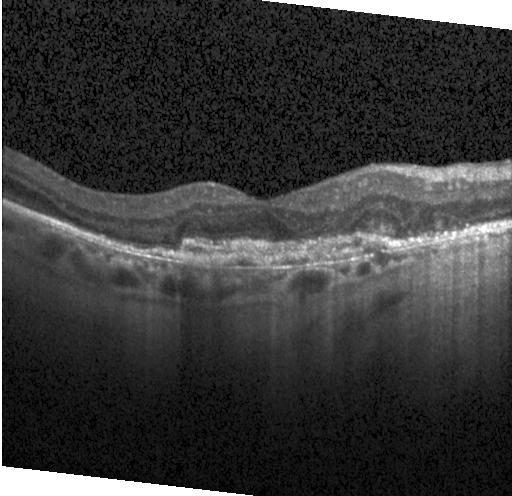 Optical coherence tomography B-scan. SD-OCT. Fovea-centered.
A choroidal neovascular membrane.